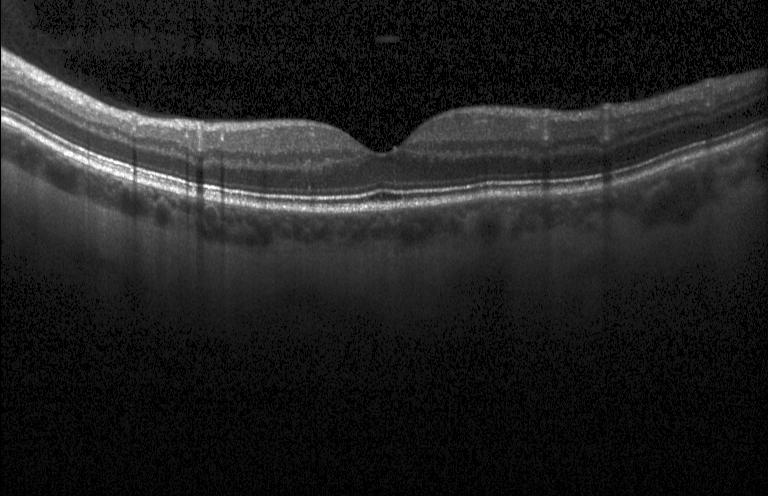

Spectral-domain optical coherence tomography. OCT line scan. Horizontal scan through the fovea
Diagnosis: neither CNV, DME, nor drusen.